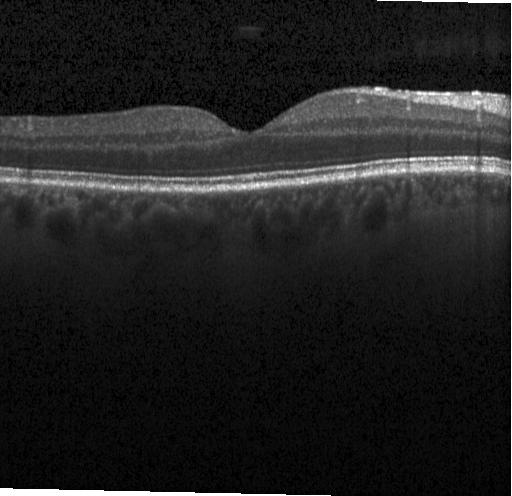 Impression: no evidence of choroidal neovascularization, diabetic macular edema, or drusen.